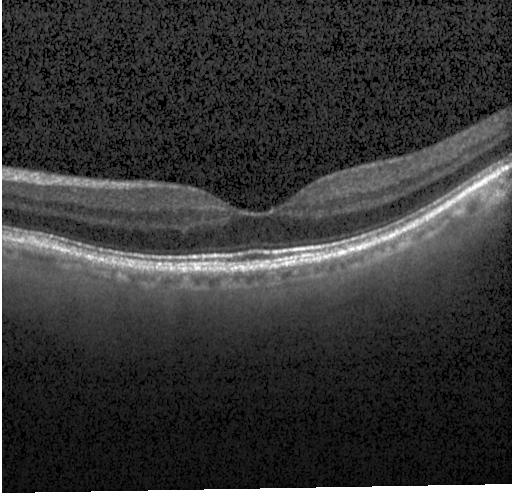
OCT line scan. SD-OCT
Impression: no evidence of choroidal neovascularization, diabetic macular edema, or drusen.